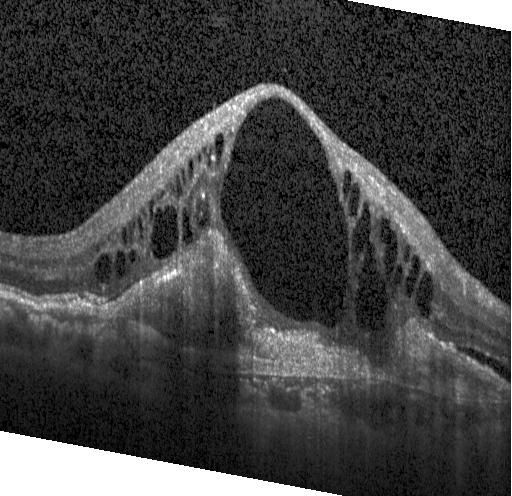
Impression: a choroidal neovascular membrane.